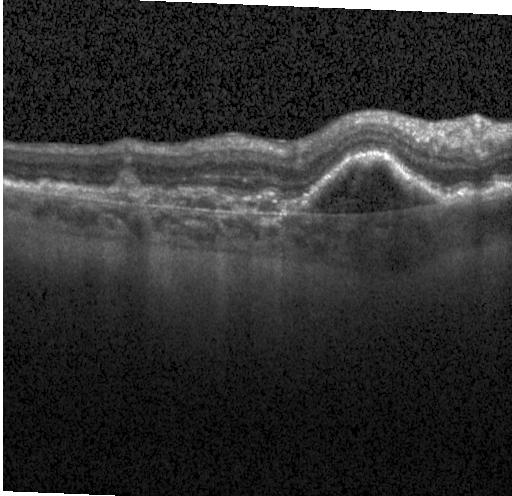 OCT line scan · instrument: Heidelberg Spectralis. Finding: choroidal neovascularization (CNV).